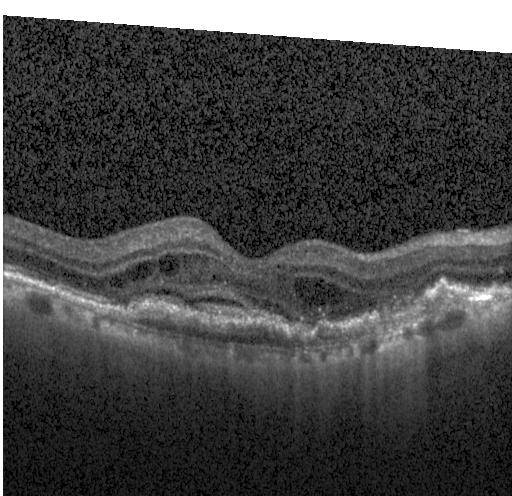

Finding: choroidal neovascularization.